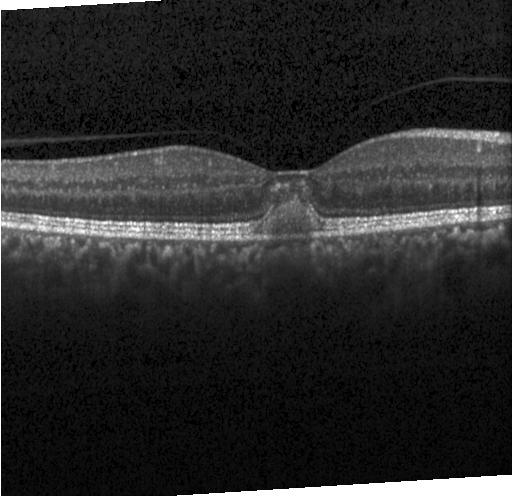

Retinal OCT cross-section
OCT finding: a choroidal neovascular membrane.